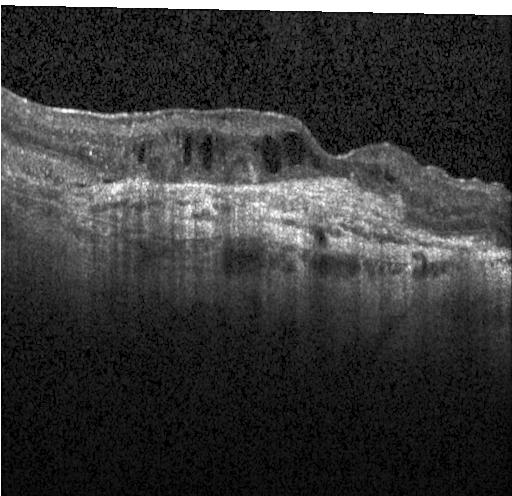
Optical coherence tomography scan · through the macula — Dx: a choroidal neovascular membrane.